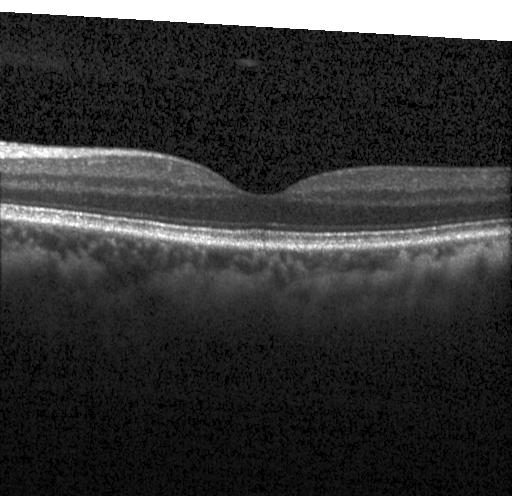 Impression: no choroidal neovascularization, no diabetic macular edema, and no drusen.